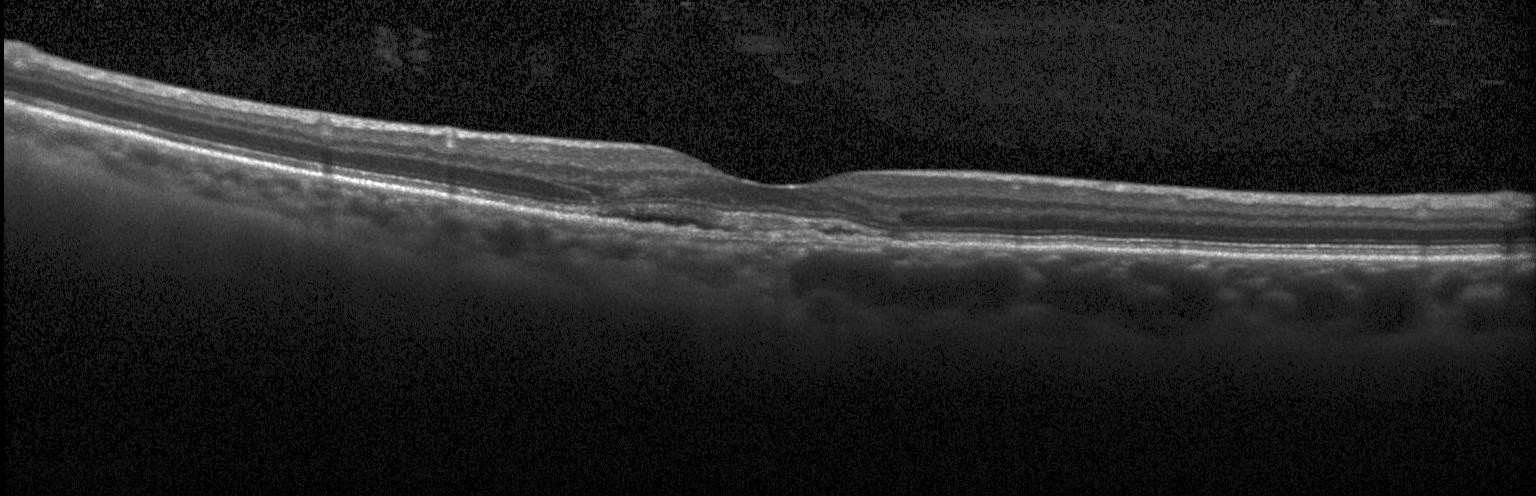 Optical coherence tomography scan, acquired on a Heidelberg Spectralis, spectral-domain OCT. OCT finding: choroidal neovascularization (CNV).